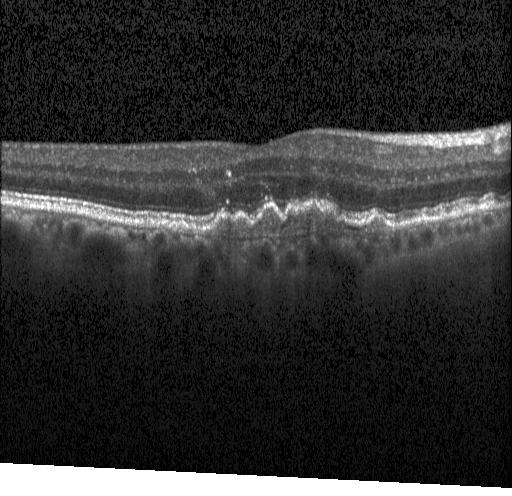 Diagnosis: a choroidal neovascular membrane.